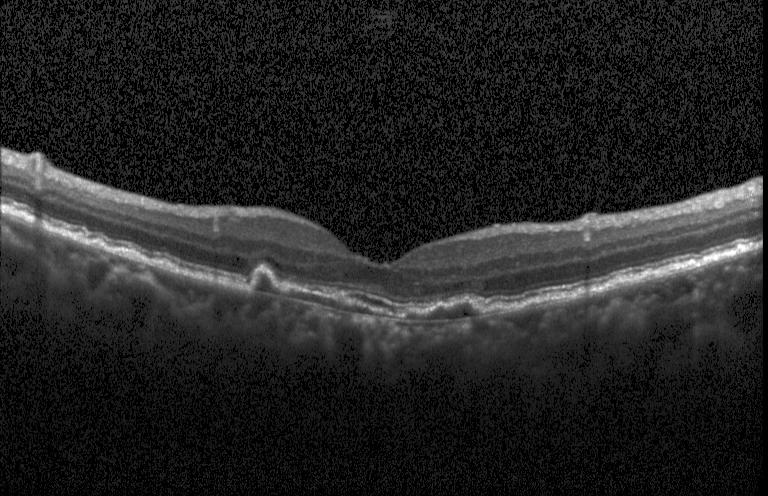 Macular scan; OCT B-scan. Impression: a choroidal neovascular membrane.